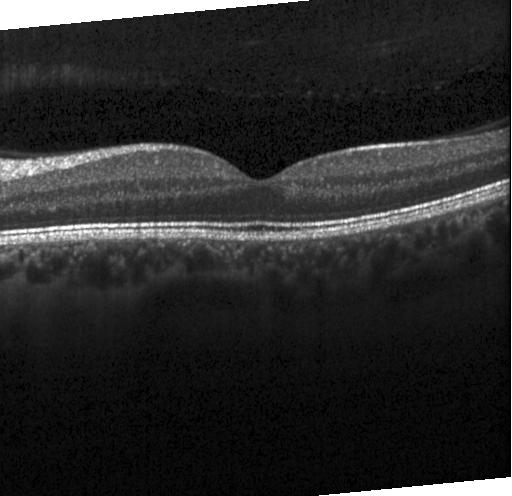
Horizontal scan through the fovea, SD-OCT, optical coherence tomography scan, instrument: Heidelberg Spectralis.
Neither CNV, DME, nor drusen.